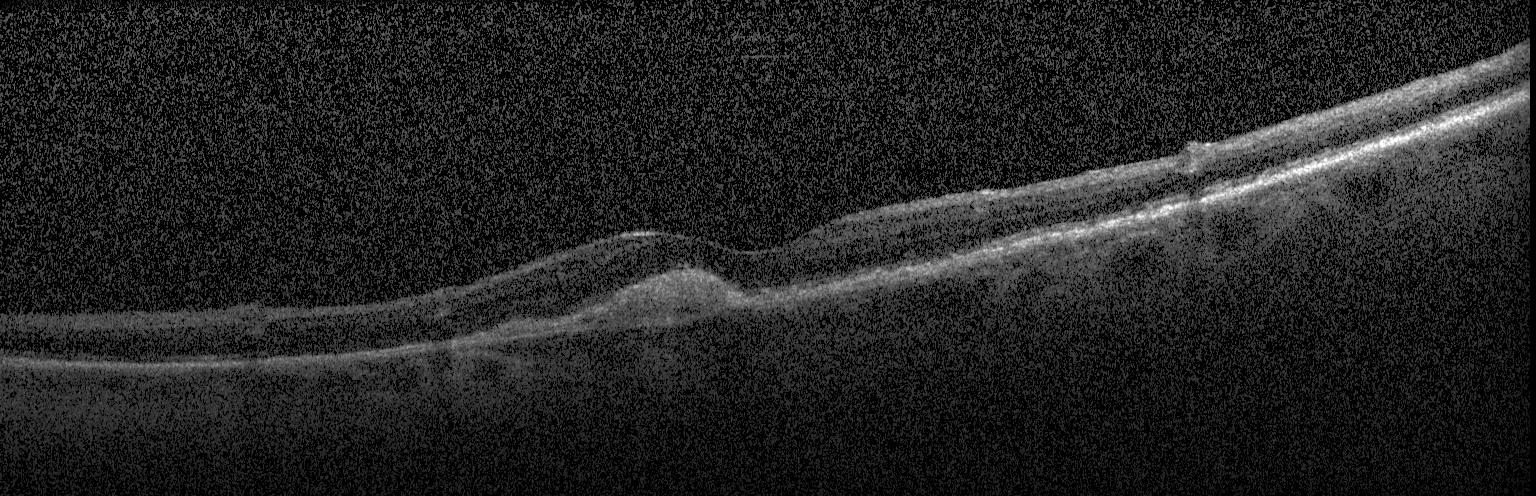

Optical coherence tomography B-scan. Diagnosis: choroidal neovascularization (CNV).